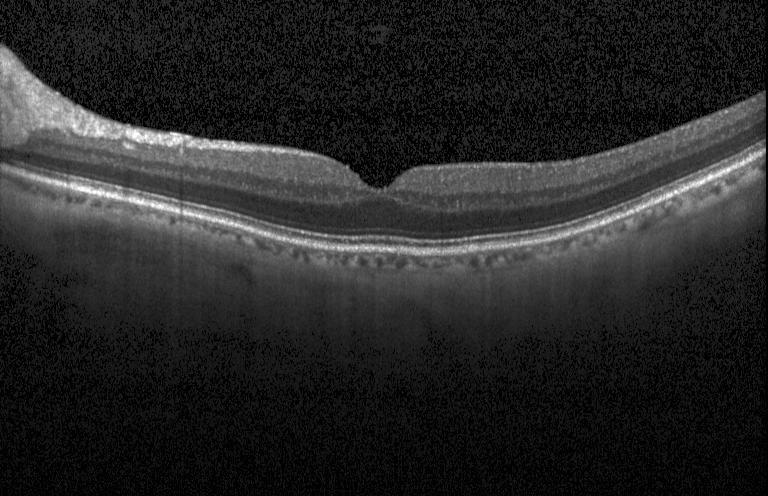 Heidelberg Spectralis OCT system; through the macula; retinal OCT B-scan — This B-scan demonstrates no choroidal neovascularization, diabetic macular edema, or drusen.